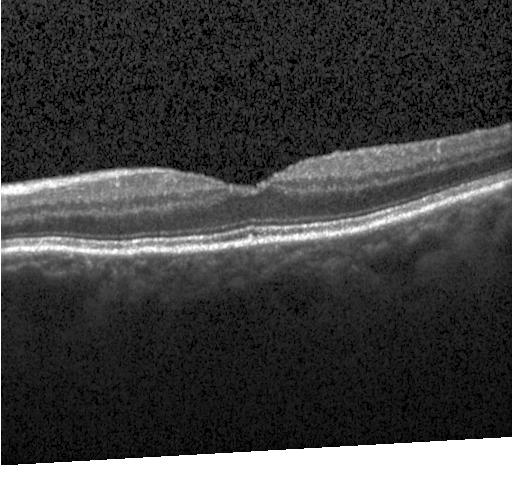 OCT scan showing neither CNV, DME, nor drusen.